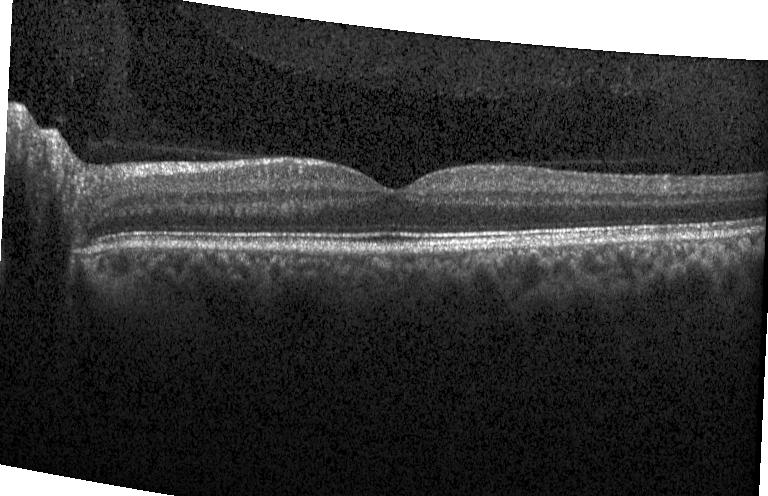 Spectral-domain OCT · optical coherence tomography scan · horizontal scan through the fovea · Heidelberg Spectralis.
Impression: no choroidal neovascularization, diabetic macular edema, or drusen.